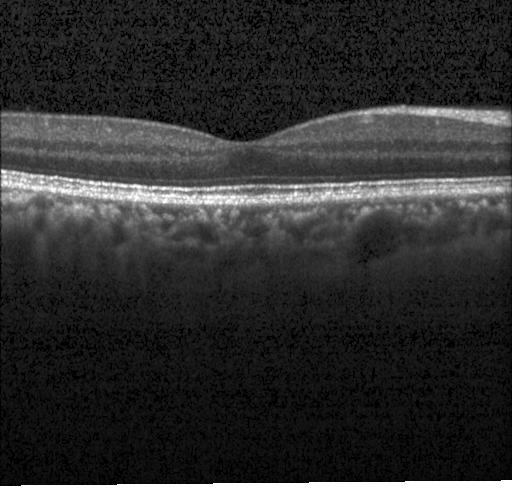 Neither CNV, DME, nor drusen.